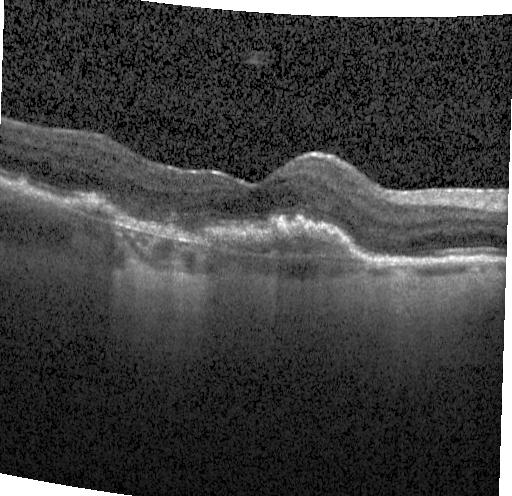

Horizontal scan through the fovea, retinal OCT cross-section — This B-scan demonstrates CNV.